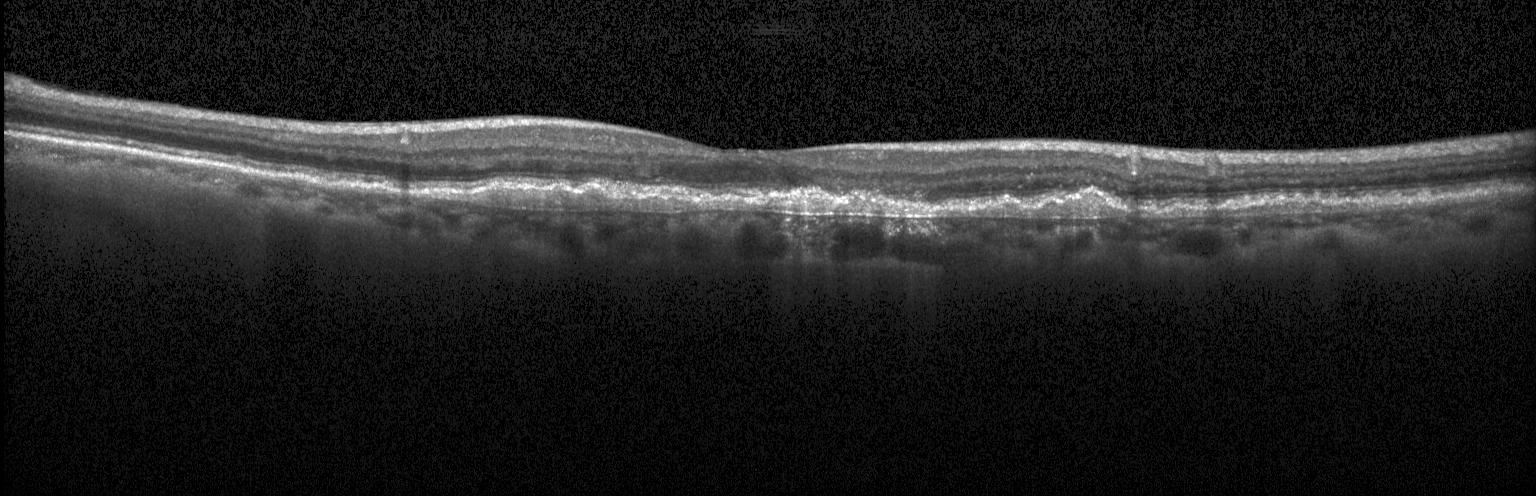 Spectral-domain OCT, OCT line scan.
CNV.